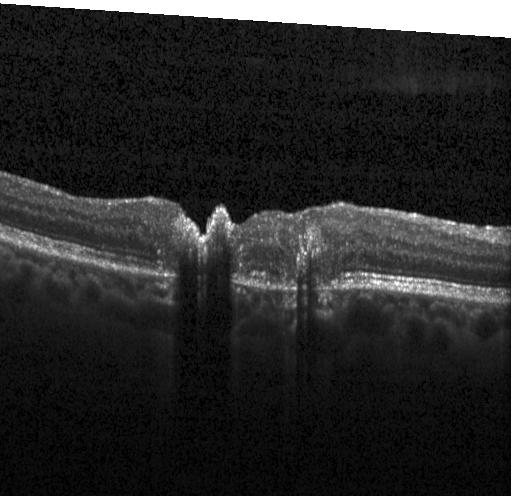
Dx: choroidal neovascularization.